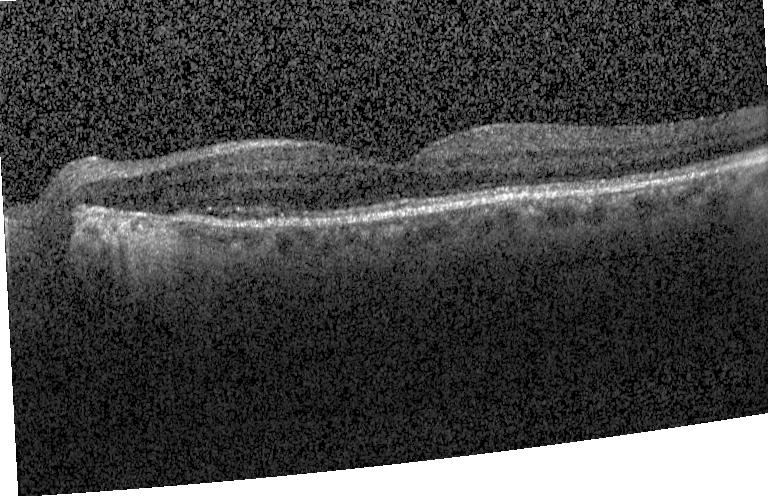

Horizontal scan through the fovea, Heidelberg Spectralis, retinal OCT B-scan.
Neither CNV, DME, nor drusen.